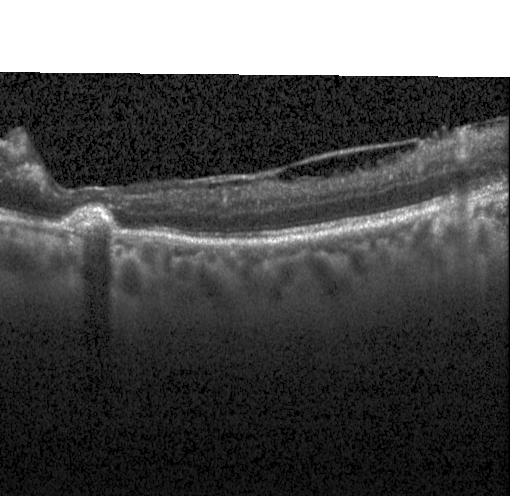 This B-scan demonstrates a choroidal neovascular membrane.